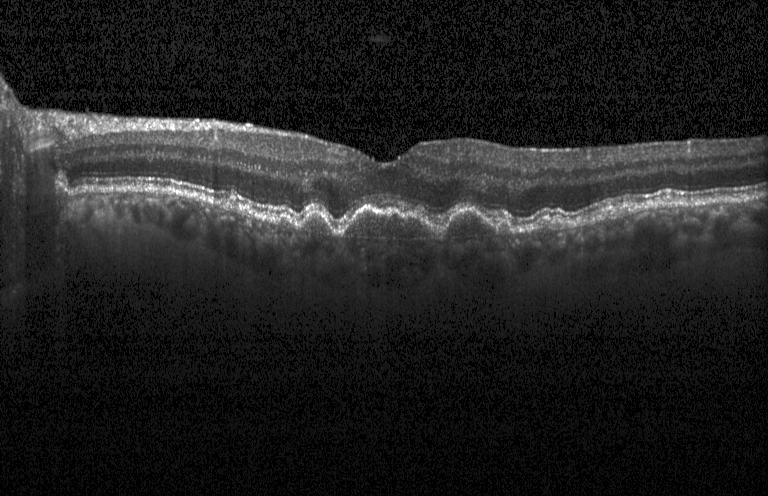 Optical coherence tomography scan. Spectral-domain OCT. Heidelberg Spectralis OCT system
Finding: sub-RPE drusenoid deposits.